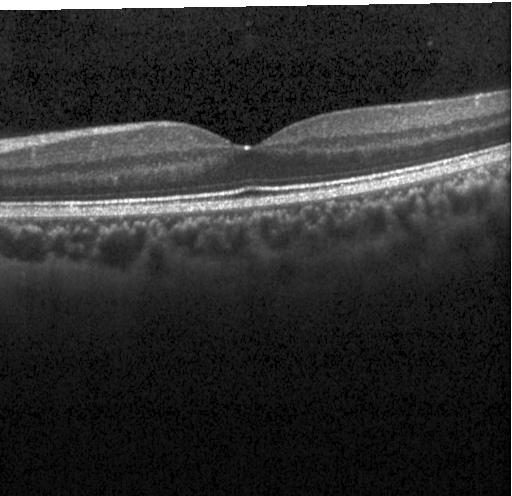 The scan shows no CNV, no DME, and no drusen.